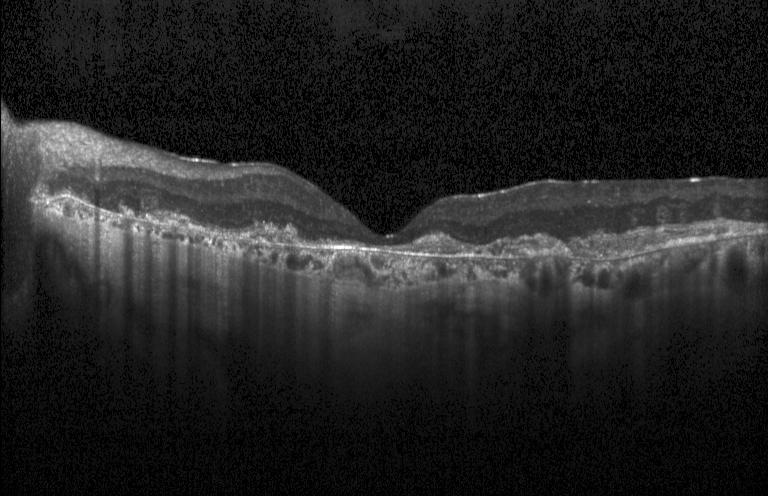 Heidelberg Spectralis; spectral-domain optical coherence tomography; retinal OCT B-scan — Choroidal neovascularization.